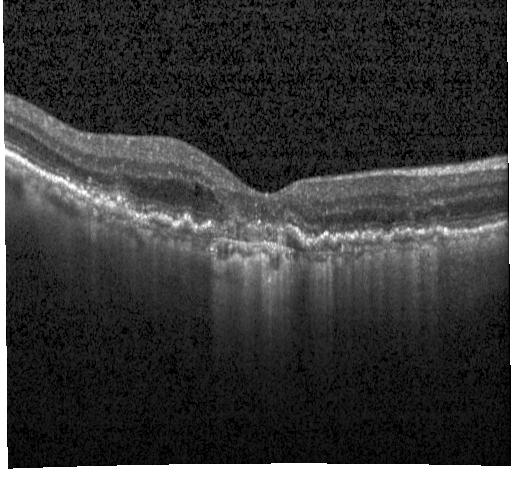

Impression: a choroidal neovascular membrane.